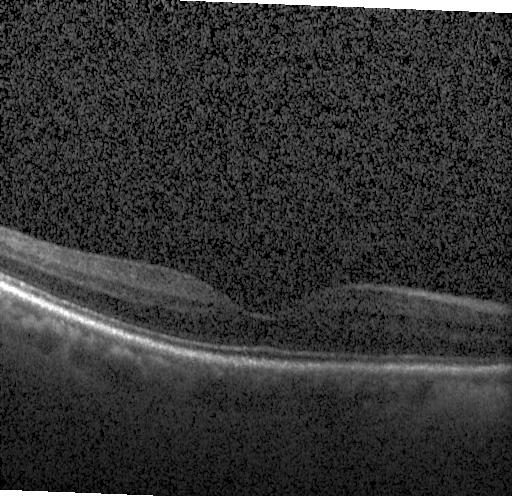
Dx: no CNV, DME, or drusen.